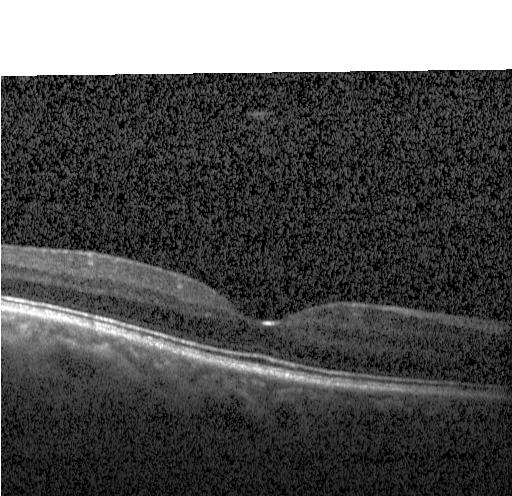 Optical coherence tomography B-scan. Dx: no choroidal neovascularization, diabetic macular edema, or drusen.